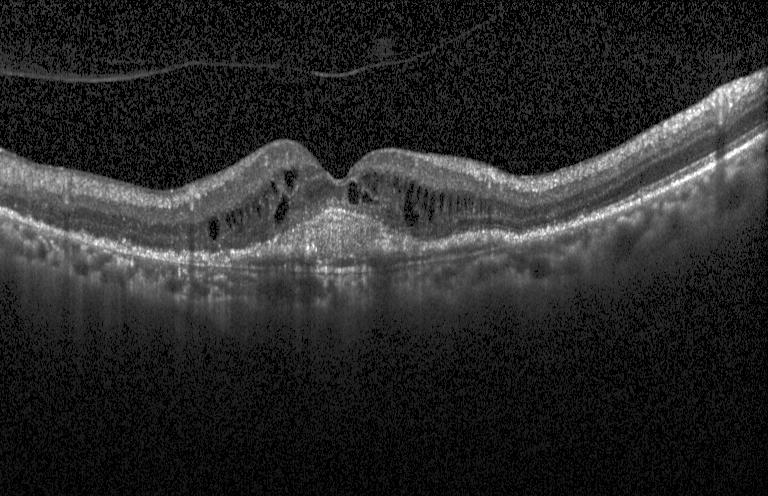

Dx: a choroidal neovascular membrane.